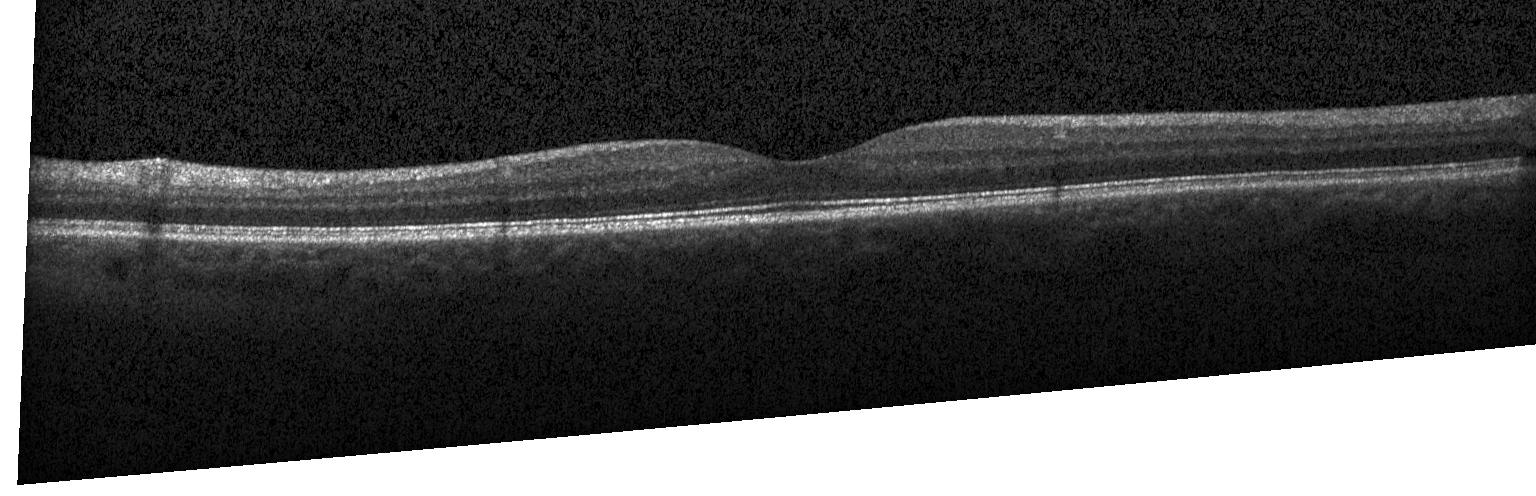
Horizontal scan through the fovea, spectral-domain OCT, optical coherence tomography scan.
Assessment: no CNV, no DME, and no drusen.